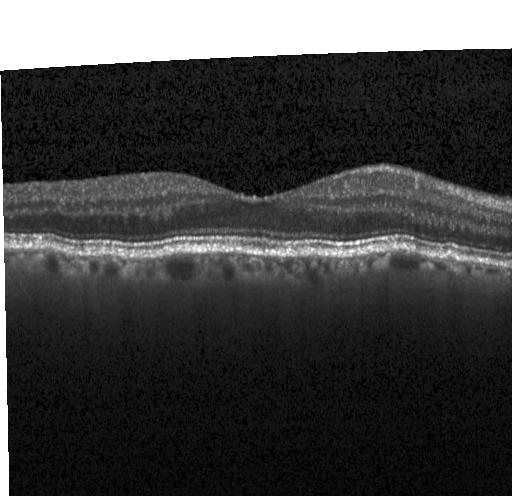

Heidelberg Spectralis. OCT line scan. Macular OCT: no CNV, DME, or drusen.